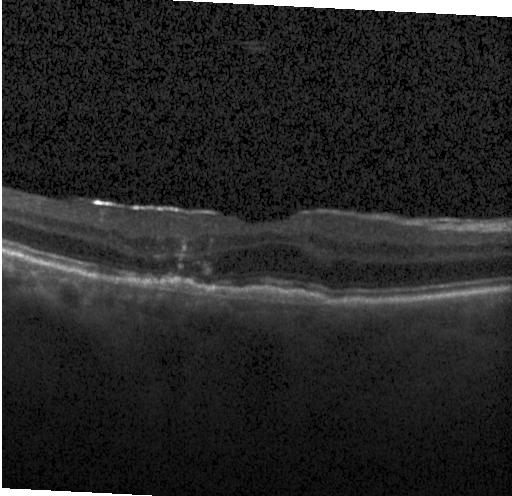
Fovea-centered, OCT line scan.
A choroidal neovascular membrane.